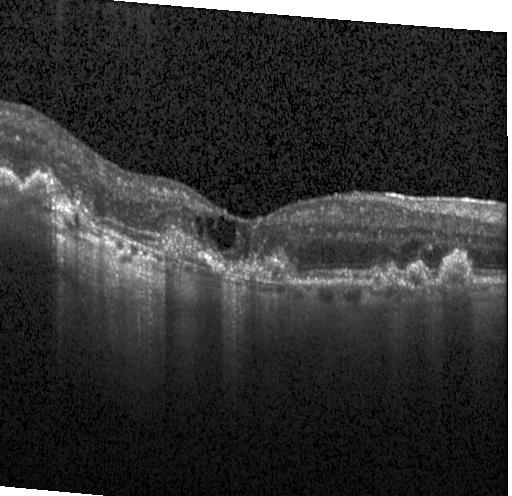
Retinal OCT B-scan, fovea-centered, acquired on a Heidelberg Spectralis, spectral-domain optical coherence tomography.
Diagnosis: a choroidal neovascular membrane.